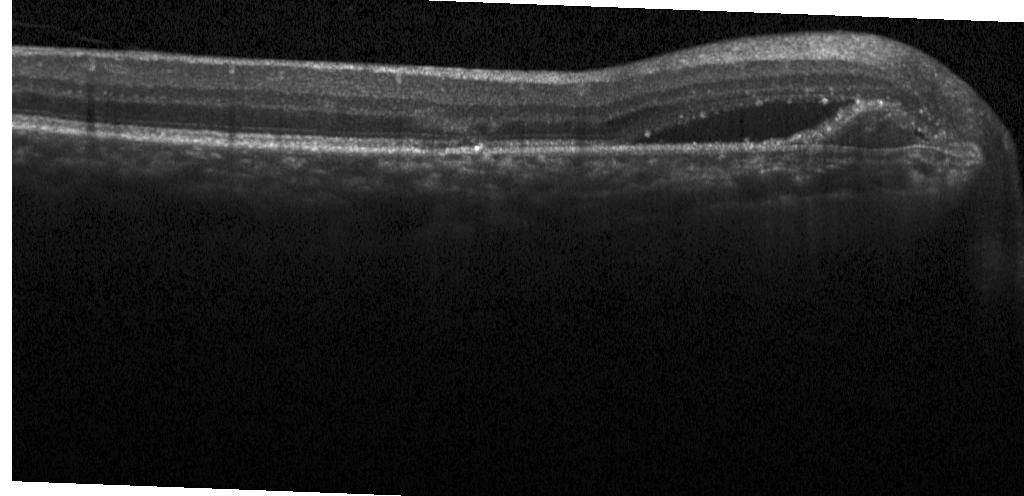
SD-OCT · retinal OCT B-scan — OCT finding: a choroidal neovascular membrane.